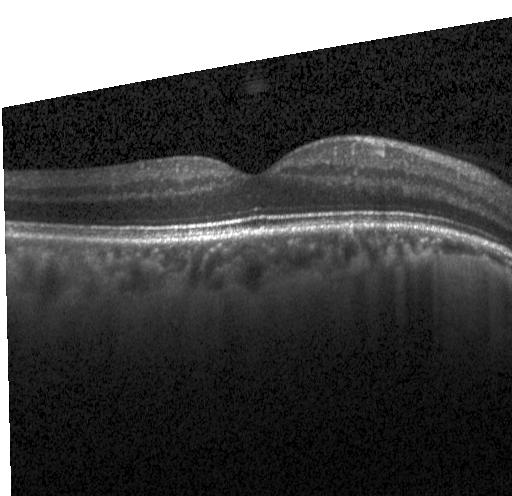
Horizontal scan through the fovea. Acquired on a Heidelberg Spectralis. OCT line scan
Finding: neither CNV, DME, nor drusen.